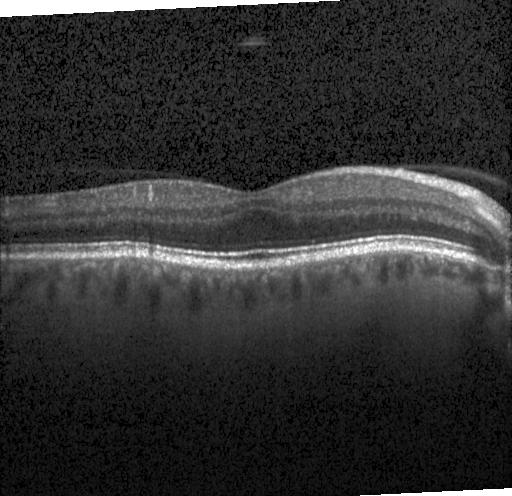 Centered on the fovea · retinal OCT cross-section.
OCT finding: no choroidal neovascularization, no diabetic macular edema, and no drusen.